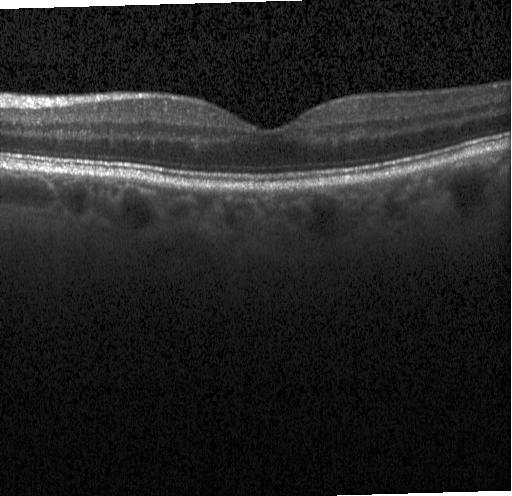
Centered on the fovea, instrument: Heidelberg Spectralis, OCT B-scan
Impression: neither CNV, DME, nor drusen.